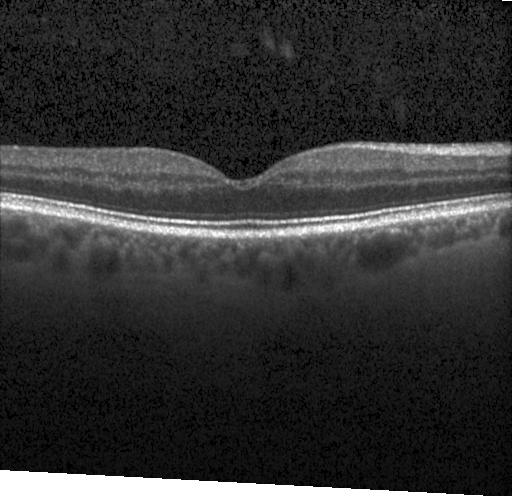
Centered on the fovea. Spectral-domain optical coherence tomography. Instrument: Heidelberg Spectralis. Optical coherence tomography scan. Finding: no choroidal neovascularization, no diabetic macular edema, and no drusen.